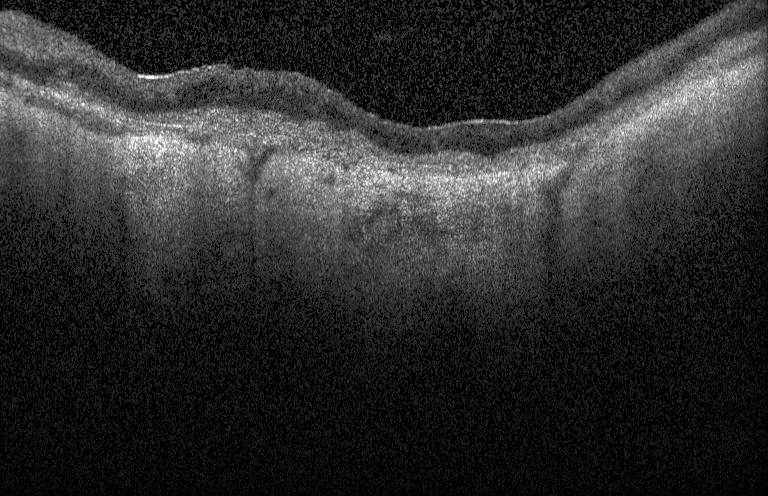
OCT line scan.
Finding: a choroidal neovascular membrane.